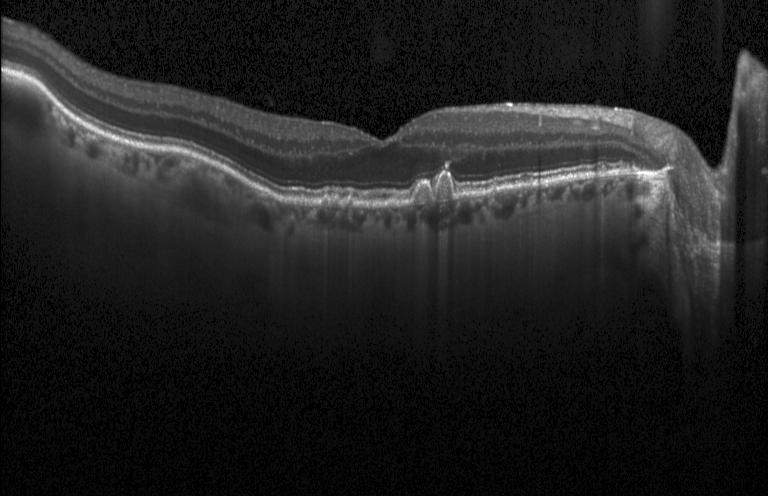
OCT B-scan; macular scan — Multiple drusen.